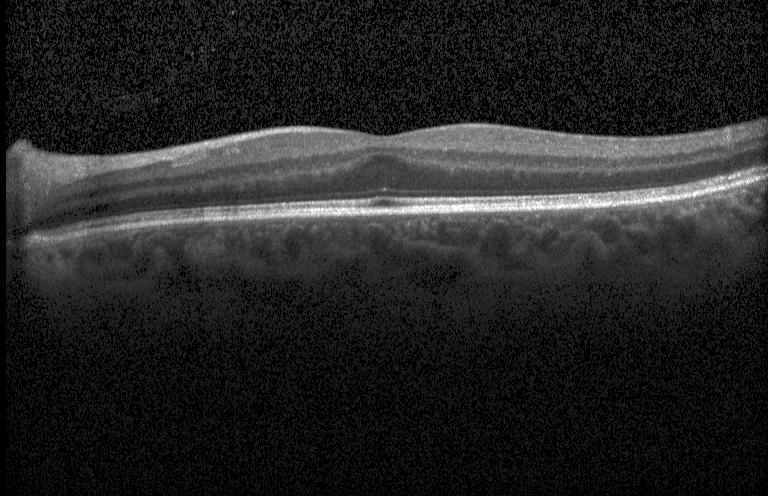
Acquired on a Heidelberg Spectralis · retinal OCT B-scan
Diagnosis: no CNV, no DME, and no drusen.